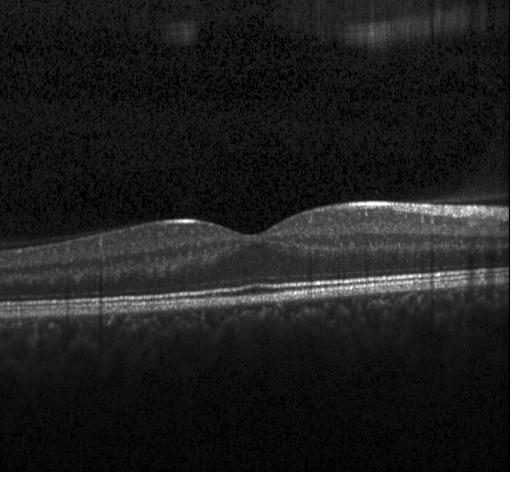

Optical coherence tomography scan — OCT finding: neither choroidal neovascularization, diabetic macular edema, nor drusen.